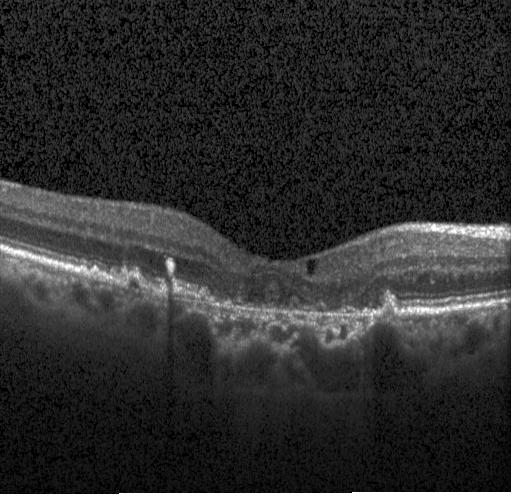 Acquired on a Heidelberg Spectralis; retinal OCT B-scan — Macular OCT: CNV.